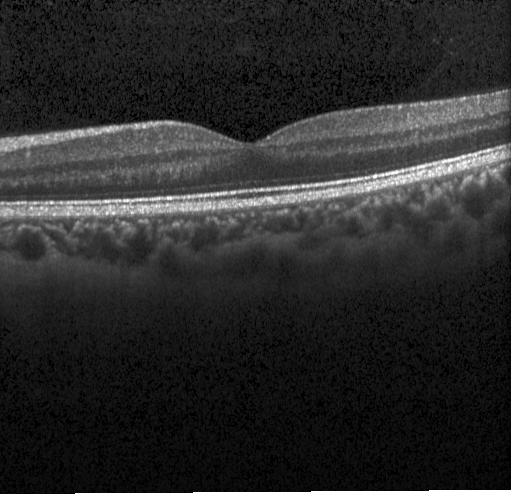
OCT B-scan. Fovea-centered.
OCT finding: no choroidal neovascularization, diabetic macular edema, or drusen.